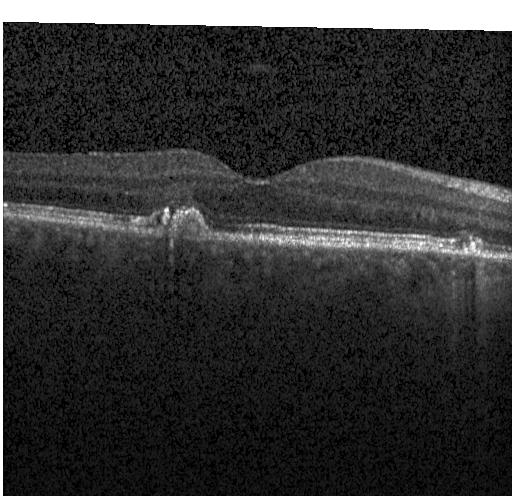
Diagnosis: a choroidal neovascular membrane.